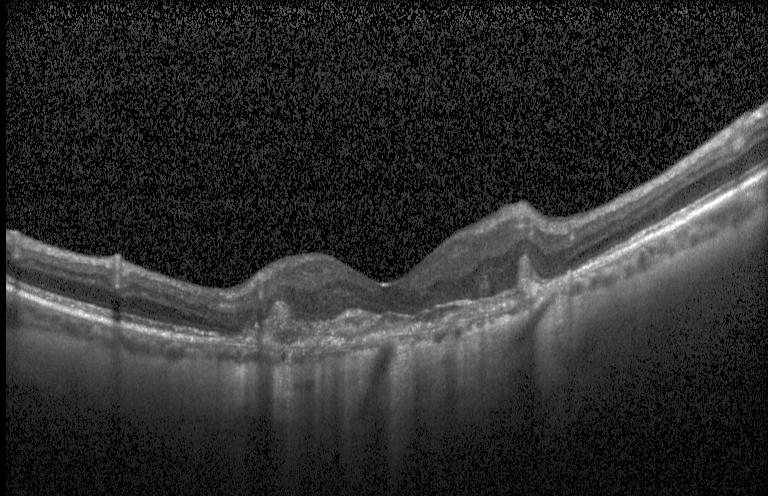
Optical coherence tomography scan; spectral-domain OCT; horizontal scan through the fovea
A choroidal neovascular membrane.